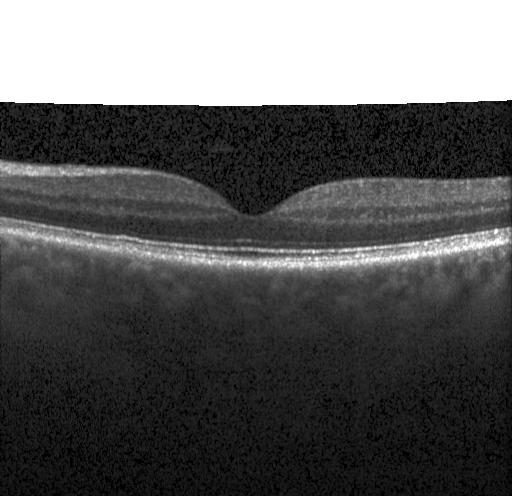

Diagnosis: neither CNV, DME, nor drusen.